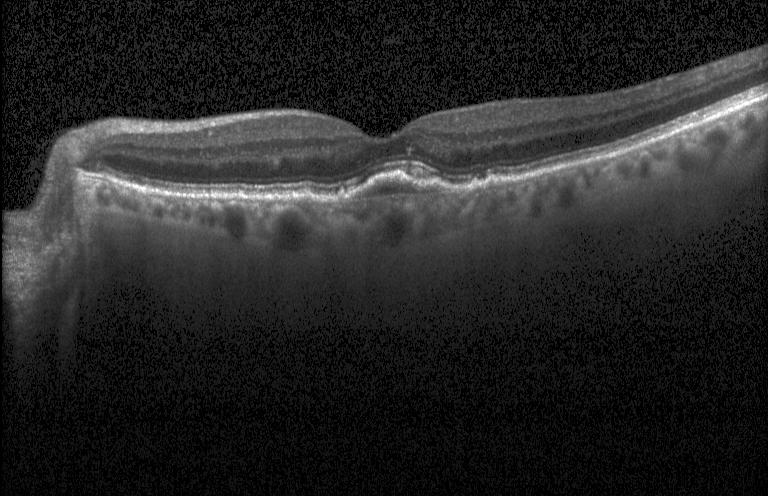
The scan shows CNV.